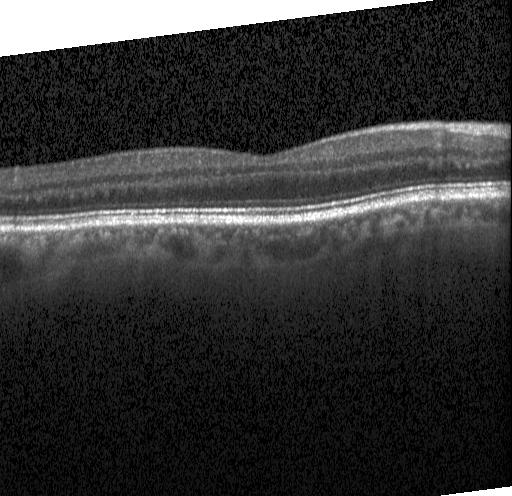

Through the macula; OCT line scan. Macular OCT: no evidence of choroidal neovascularization, diabetic macular edema, or drusen.